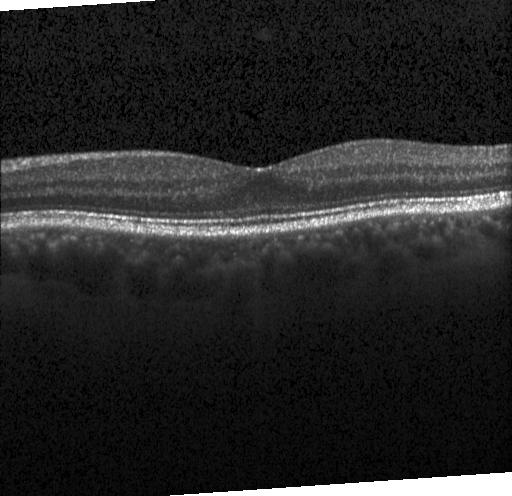

Optical coherence tomography B-scan. SD-OCT. Centered on the fovea. Instrument: Heidelberg Spectralis.
Neither choroidal neovascularization, diabetic macular edema, nor drusen.